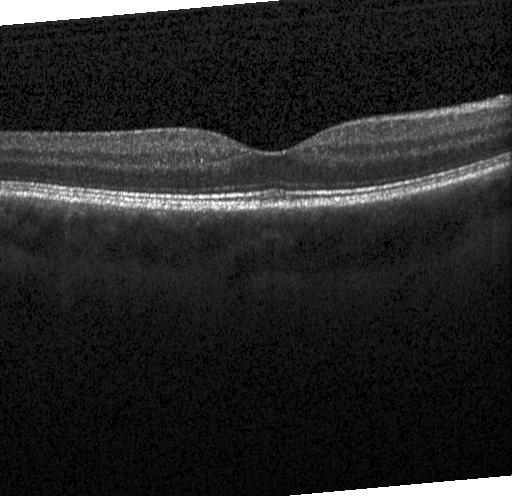

Diagnosis: no choroidal neovascularization, diabetic macular edema, or drusen.